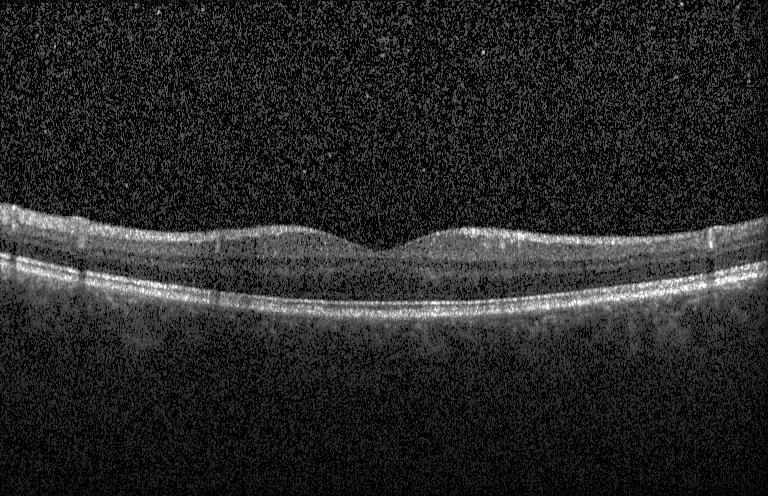
Horizontal scan through the fovea. SD-OCT. Optical coherence tomography scan.
Impression: neither choroidal neovascularization, diabetic macular edema, nor drusen.